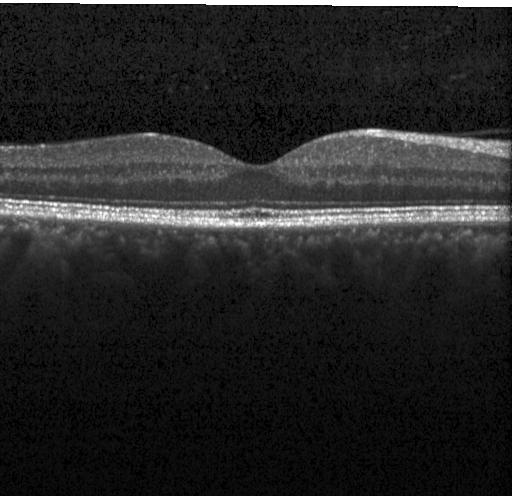

Optical coherence tomography scan — Diagnosis: no evidence of choroidal neovascularization, diabetic macular edema, or drusen.